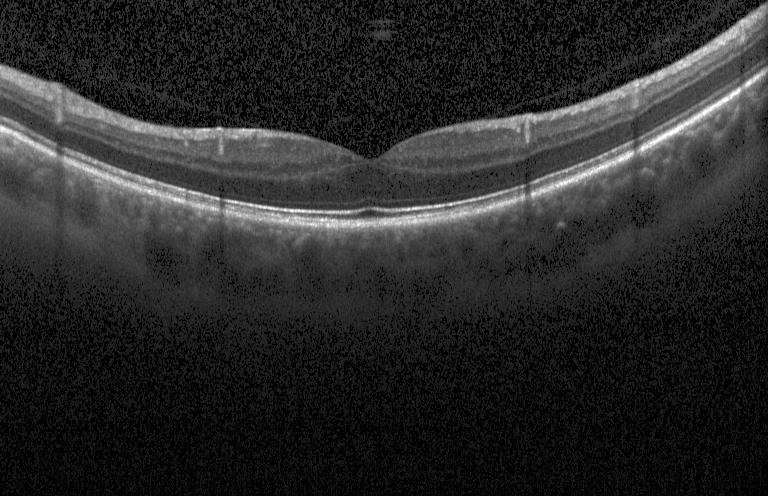 Heidelberg Spectralis OCT system, OCT line scan, horizontal scan through the fovea, spectral-domain OCT
This B-scan demonstrates no choroidal neovascularization, diabetic macular edema, or drusen.